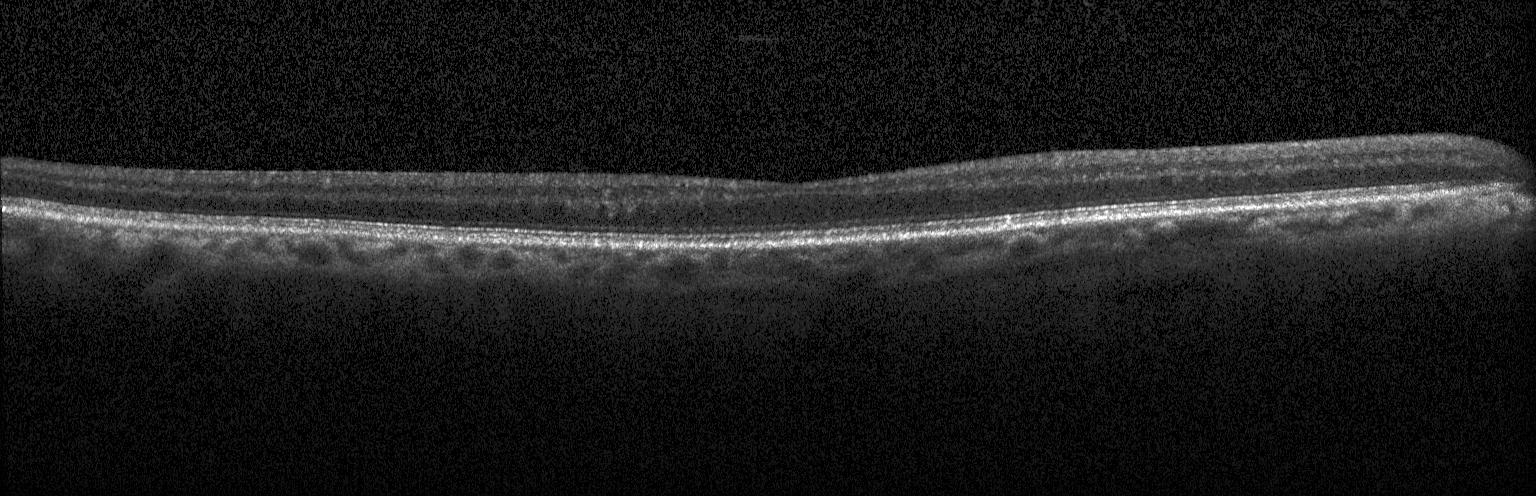

OCT finding: neither choroidal neovascularization, diabetic macular edema, nor drusen.